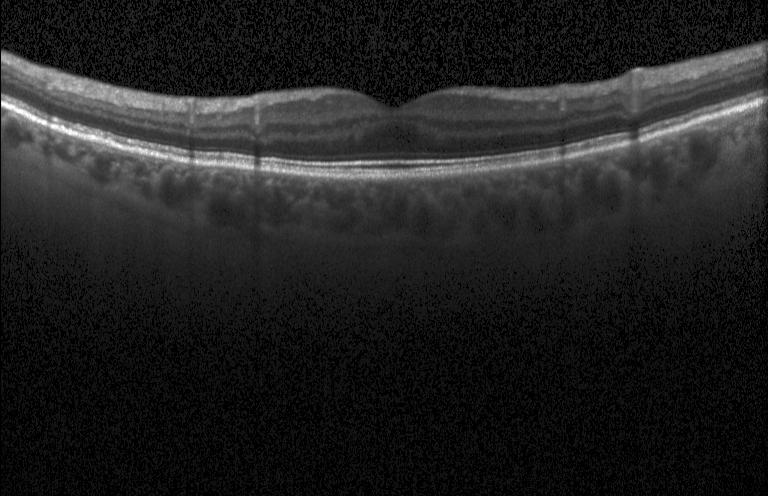 Through the macula, spectral-domain OCT, instrument: Heidelberg Spectralis, retinal OCT B-scan — No evidence of choroidal neovascularization, diabetic macular edema, or drusen.